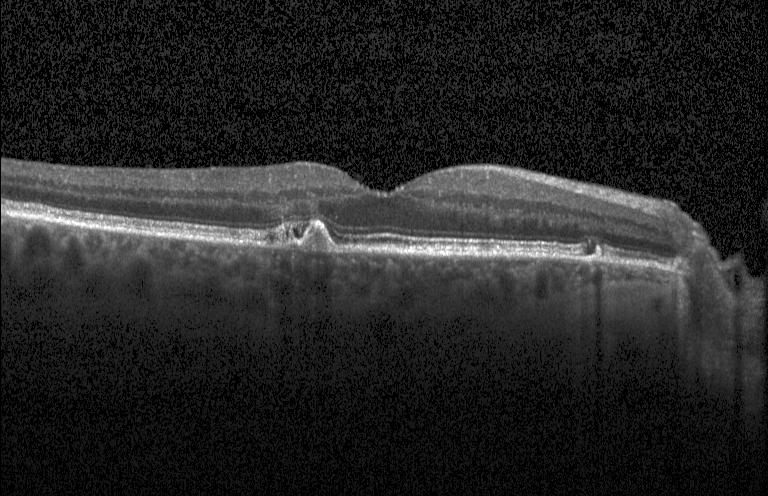

This B-scan demonstrates a choroidal neovascular membrane.